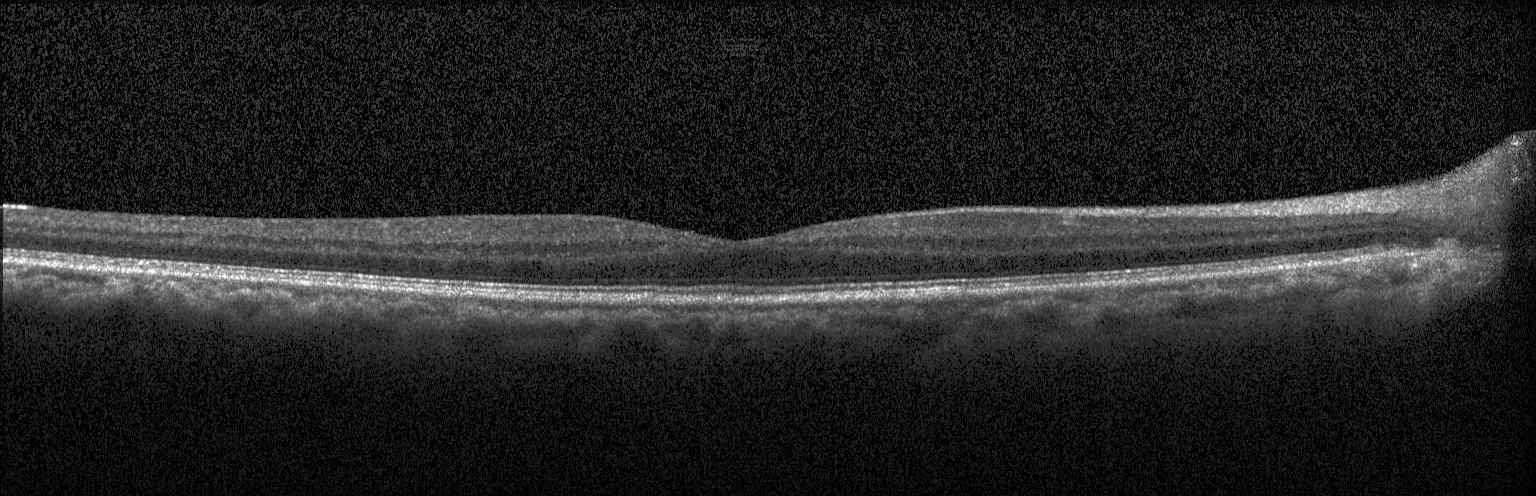

Retinal OCT B-scan.
Finding: no choroidal neovascularization, diabetic macular edema, or drusen.